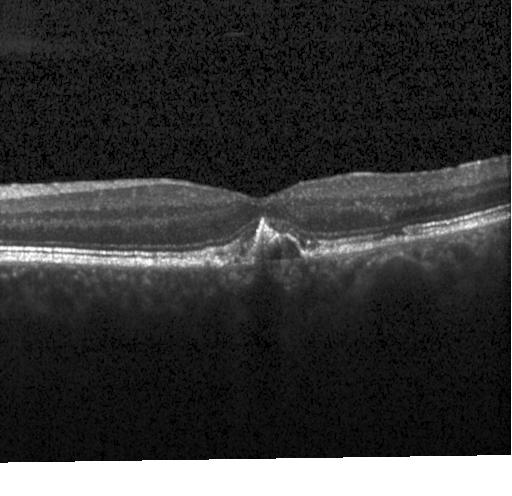 Optical coherence tomography B-scan · fovea-centered · instrument: Heidelberg Spectralis. This B-scan demonstrates CNV.